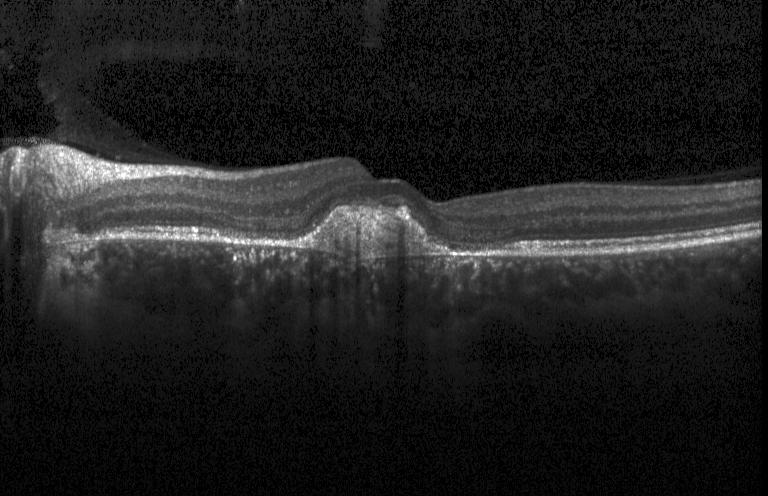

Optical coherence tomography B-scan; instrument: Heidelberg Spectralis; horizontal scan through the fovea
The scan shows choroidal neovascularization.